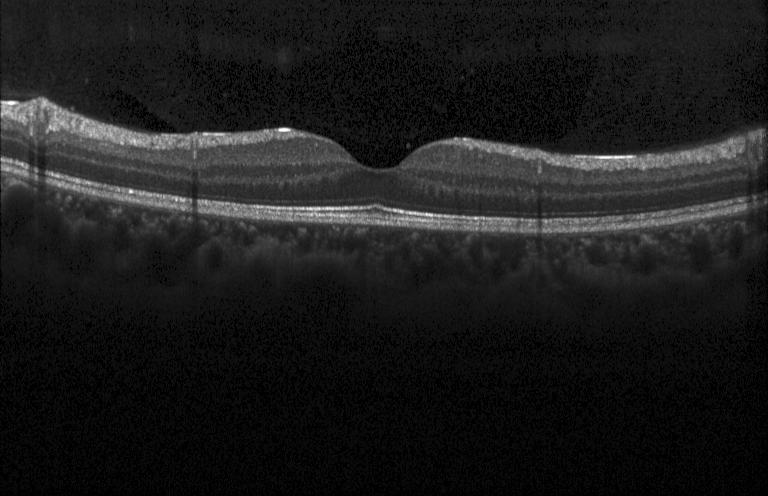 Retinal OCT B-scan
Assessment: neither CNV, DME, nor drusen.